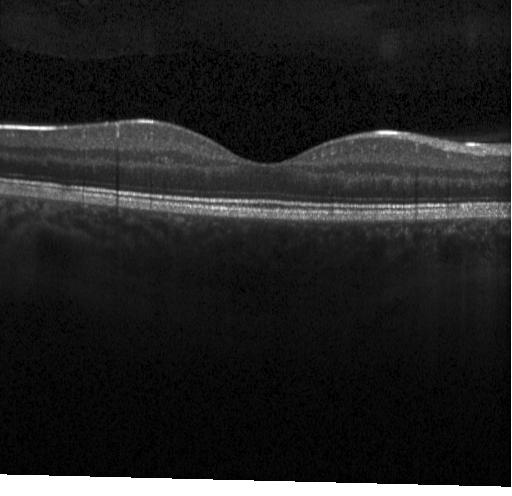 Optical coherence tomography B-scan · SD-OCT · macular scan — No choroidal neovascularization, diabetic macular edema, or drusen.